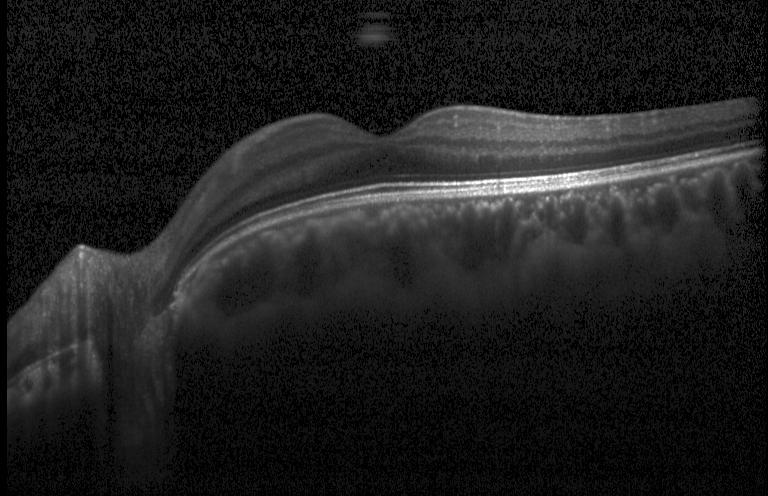

SD-OCT · optical coherence tomography scan — This B-scan demonstrates neither choroidal neovascularization, diabetic macular edema, nor drusen.